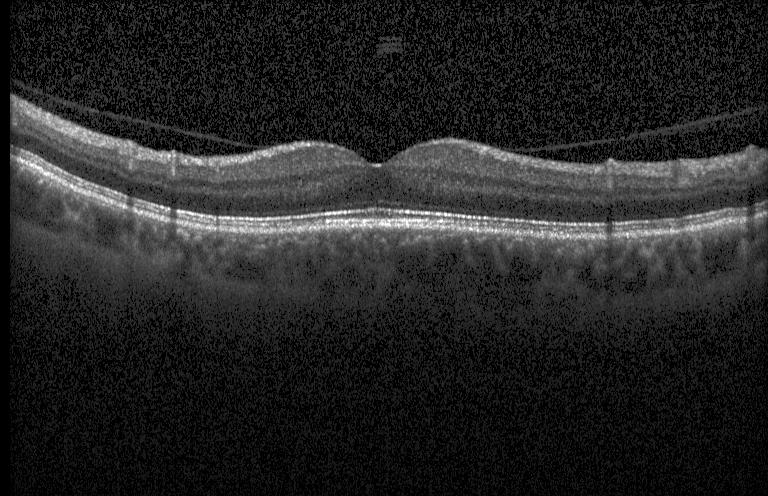 OCT B-scan showing no CNV, no DME, and no drusen.